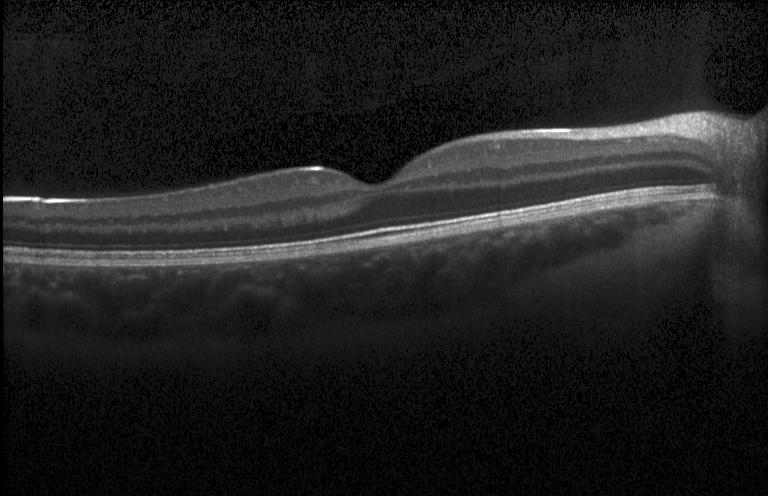

The scan shows no choroidal neovascularization, diabetic macular edema, or drusen.